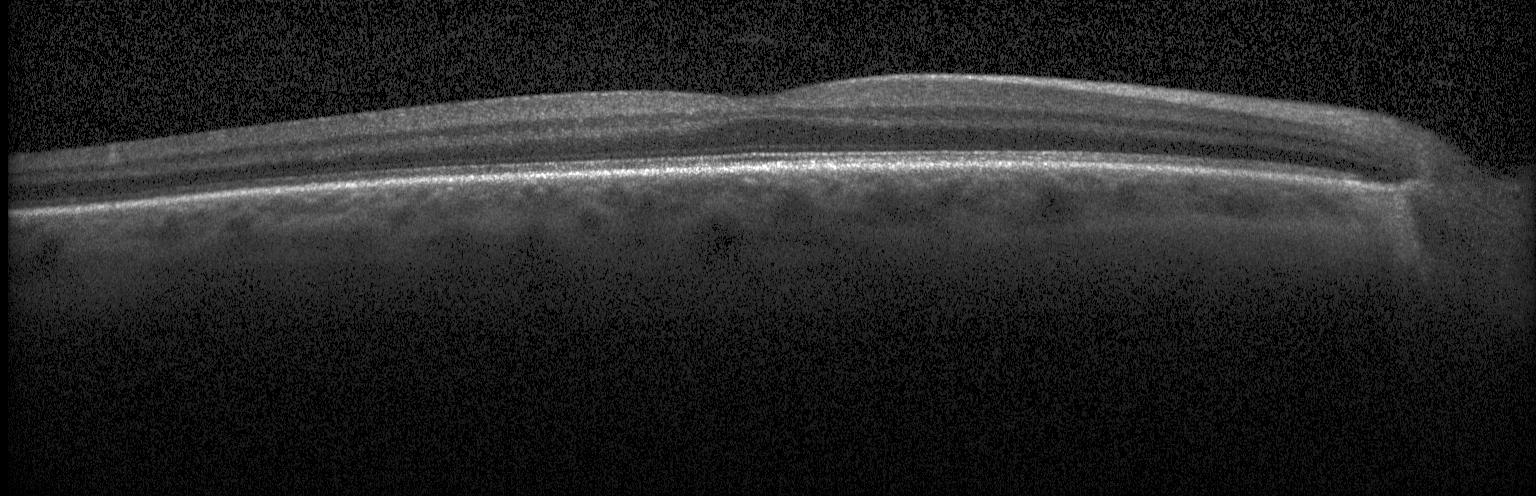

Acquired on a Heidelberg Spectralis · optical coherence tomography B-scan.
Finding: no CNV, DME, or drusen.